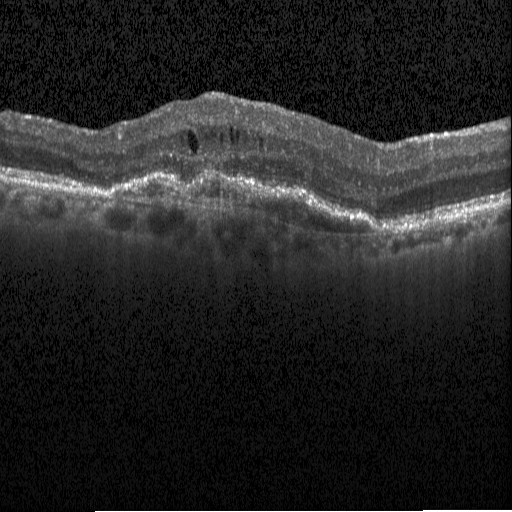
Spectral-domain OCT B-scan: DME.